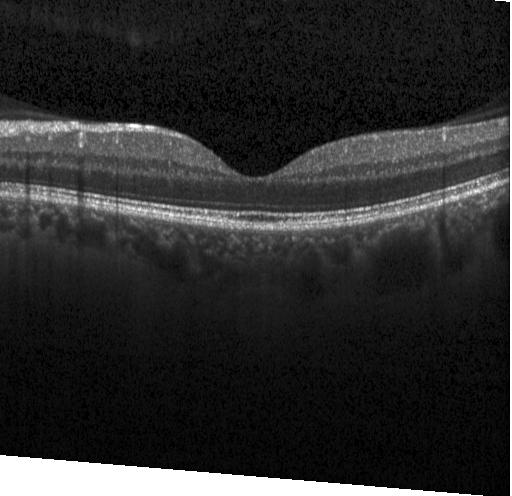

Spectral-domain OCT · instrument: Heidelberg Spectralis · fovea-centered · optical coherence tomography scan. No choroidal neovascularization, diabetic macular edema, or drusen.